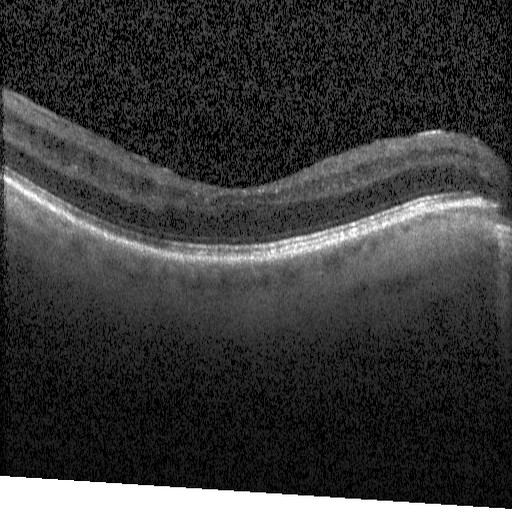 Fovea-centered; spectral-domain OCT; optical coherence tomography scan — Diagnosis: diabetic macular edema.